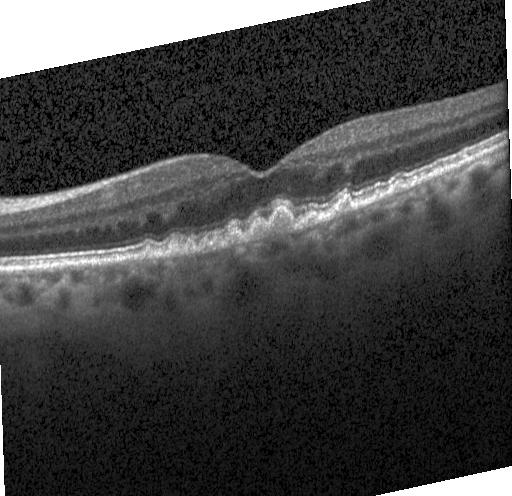
Finding: drusen.